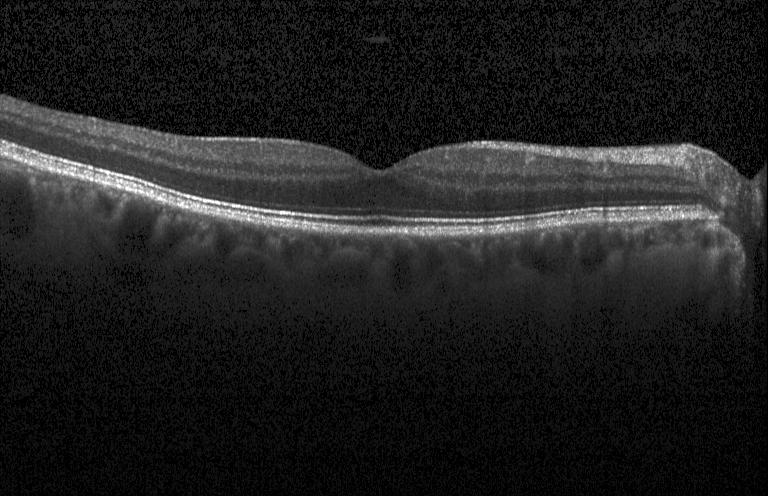
Impression: no CNV, no DME, and no drusen.